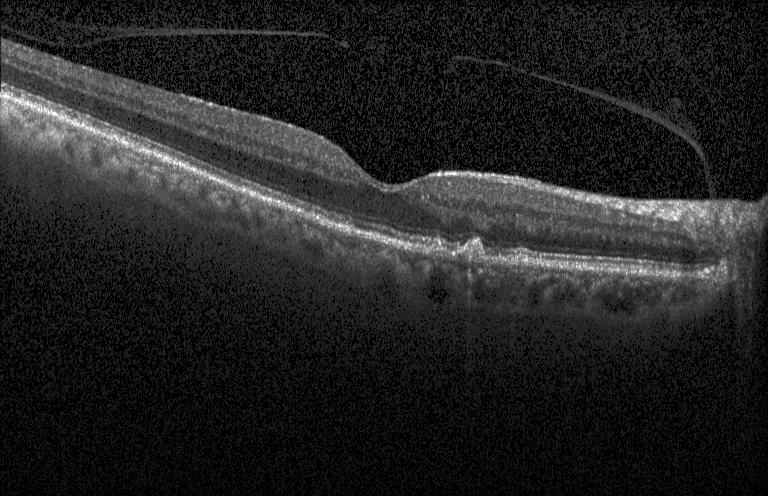

Centered on the fovea · Heidelberg Spectralis · spectral-domain OCT · optical coherence tomography B-scan. Finding: sub-RPE drusenoid deposits.